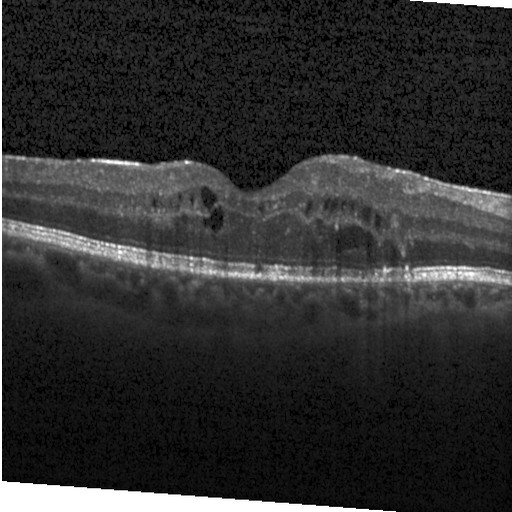
Heidelberg Spectralis OCT system. SD-OCT. Macular scan. Optical coherence tomography B-scan
Diabetic macular edema (DME).